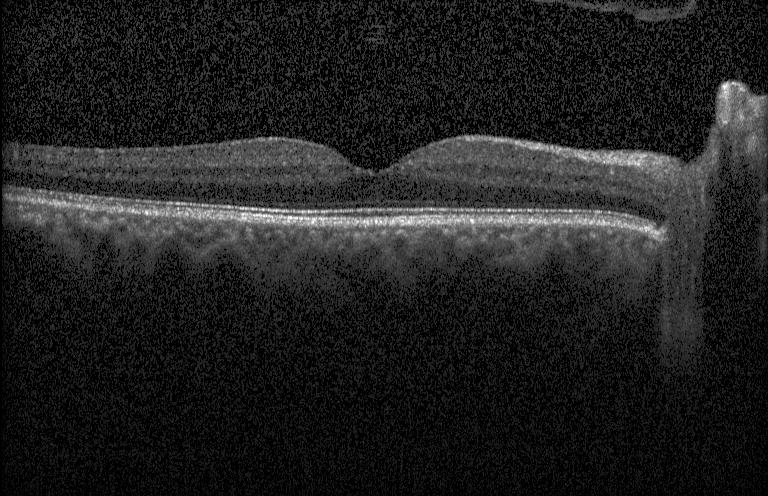

Centered on the fovea. Spectral-domain OCT. Retinal OCT cross-section. Heidelberg Spectralis — Finding: no CNV, no DME, and no drusen.